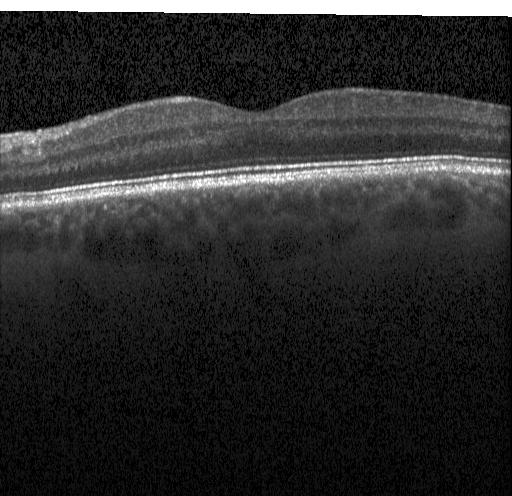

Heidelberg Spectralis OCT system · optical coherence tomography B-scan. Dx: no choroidal neovascularization, no diabetic macular edema, and no drusen.